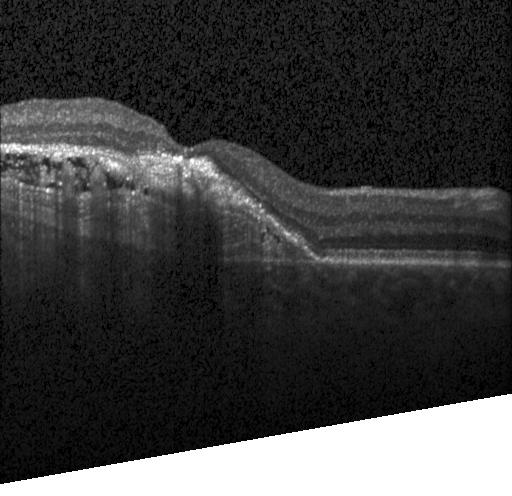 Spectral-domain OCT · retinal OCT B-scan · horizontal scan through the fovea
Finding: a choroidal neovascular membrane.